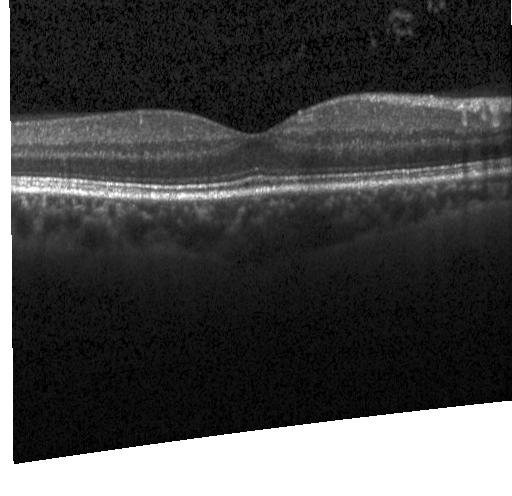 Heidelberg Spectralis OCT system; macular scan; optical coherence tomography B-scan; SD-OCT.
Finding: neither choroidal neovascularization, diabetic macular edema, nor drusen.